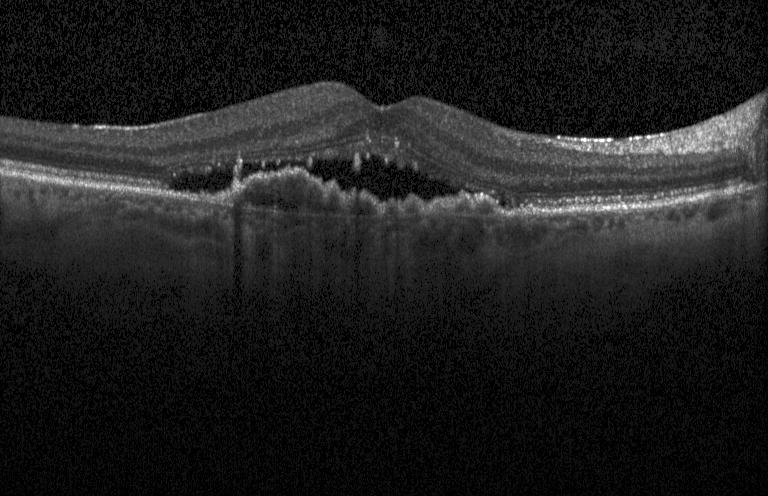
A choroidal neovascular membrane.